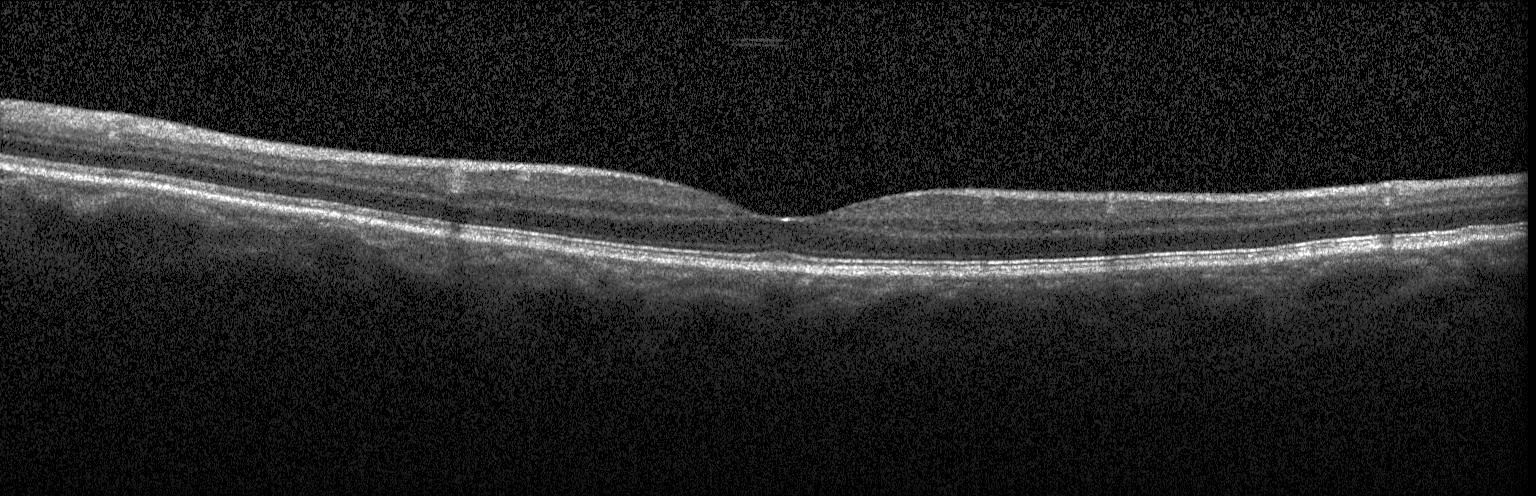

Optical coherence tomography B-scan.
OCT finding: no evidence of choroidal neovascularization, diabetic macular edema, or drusen.